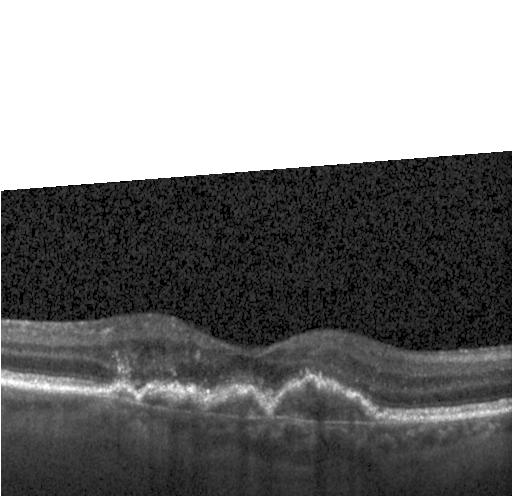 OCT line scan. Acquired on a Heidelberg Spectralis
A choroidal neovascular membrane.